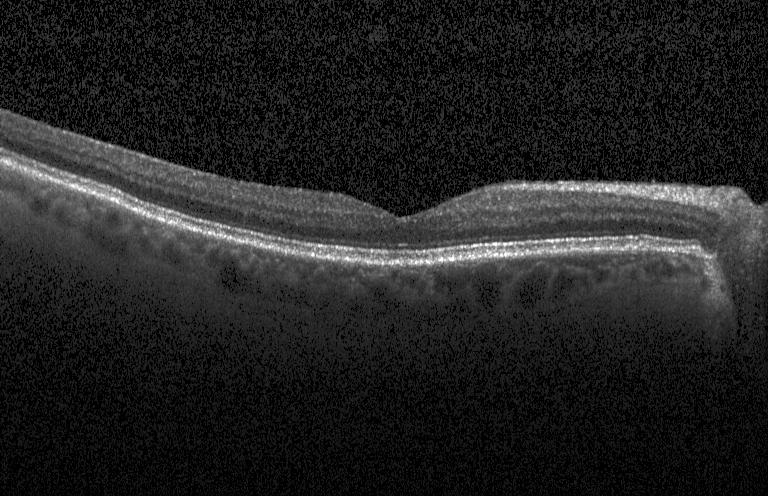

Impression: neither choroidal neovascularization, diabetic macular edema, nor drusen.